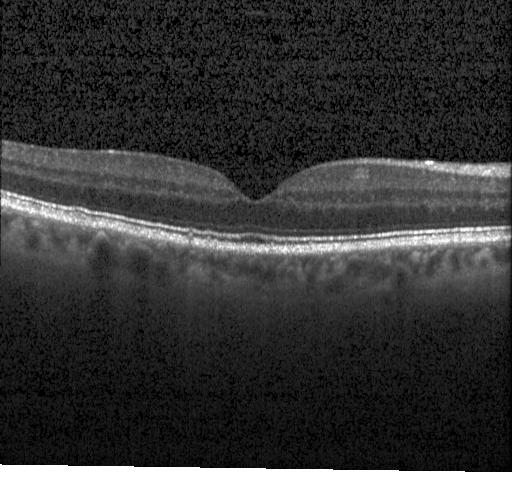 Heidelberg Spectralis OCT system; centered on the fovea; spectral-domain OCT; retinal OCT B-scan
Diagnosis: no choroidal neovascularization, diabetic macular edema, or drusen.